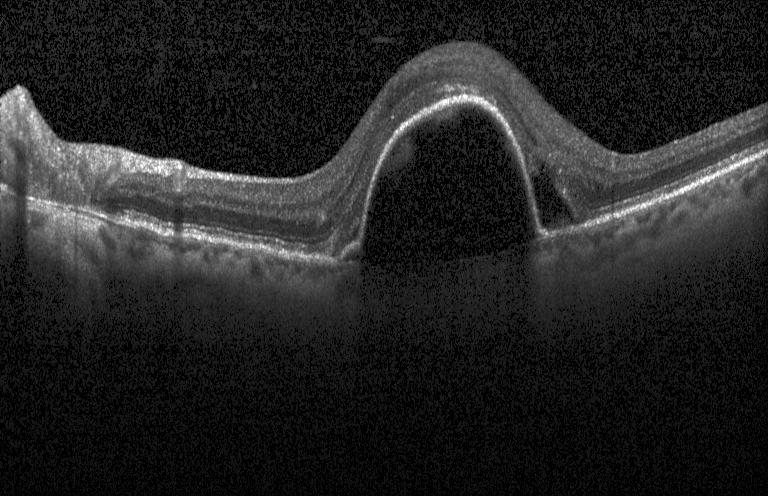

Heidelberg Spectralis, OCT line scan, centered on the fovea — Assessment: choroidal neovascularization.